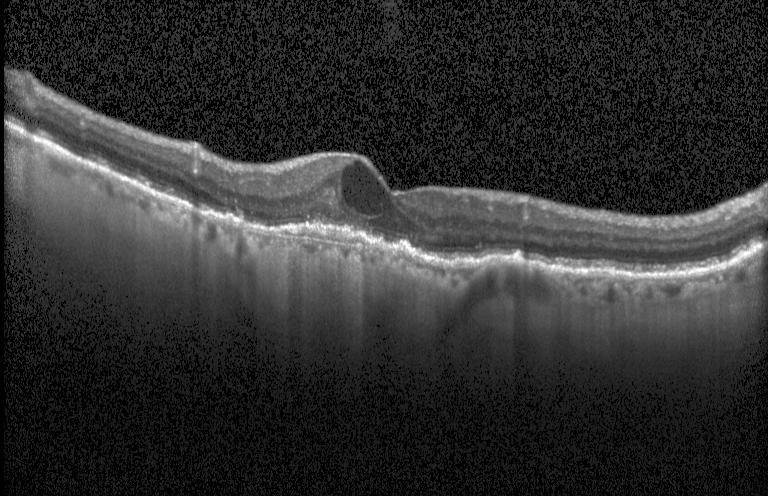 OCT line scan. Impression: choroidal neovascularization.